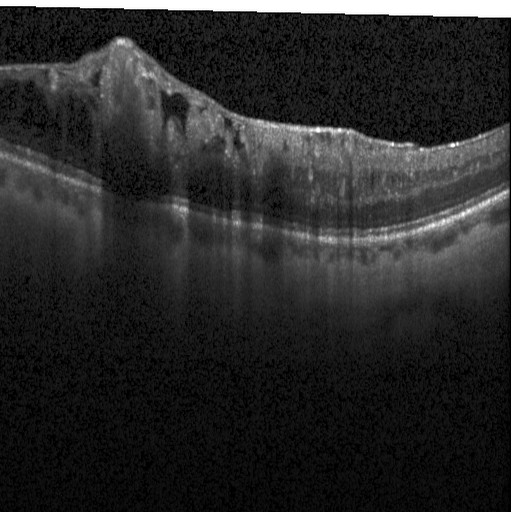 Impression: DME.